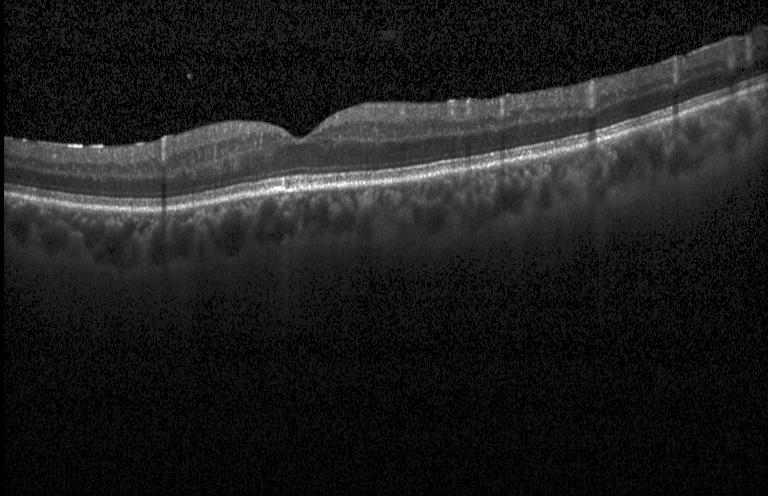
Heidelberg Spectralis OCT system; retinal OCT B-scan; fovea-centered. Diagnosis: no evidence of CNV, DME, or drusen.